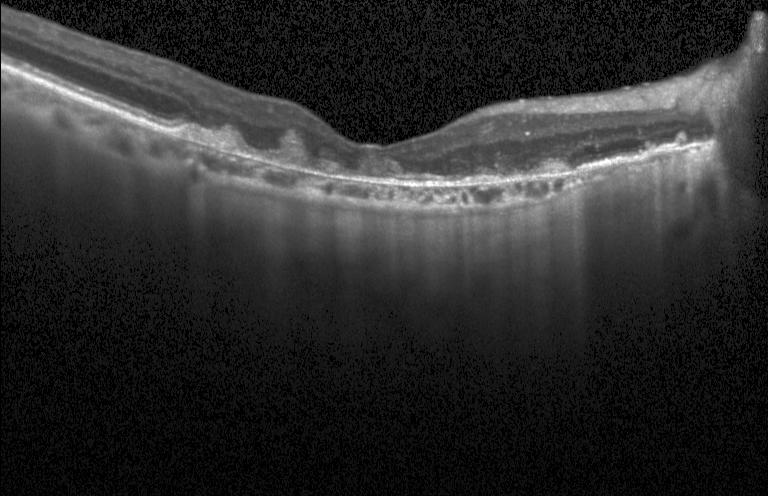
Centered on the fovea, optical coherence tomography scan — OCT finding: choroidal neovascularization.